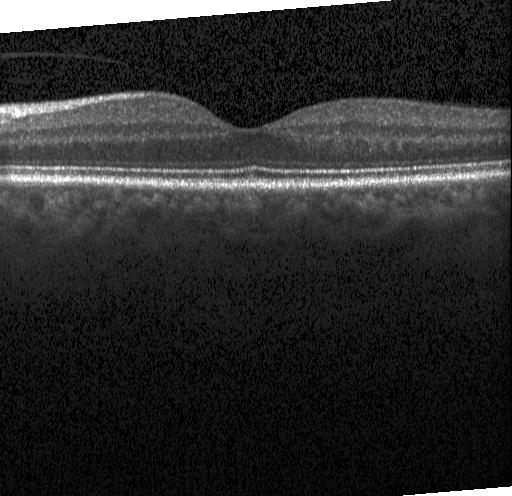

OCT line scan, SD-OCT
Macular OCT: neither choroidal neovascularization, diabetic macular edema, nor drusen.